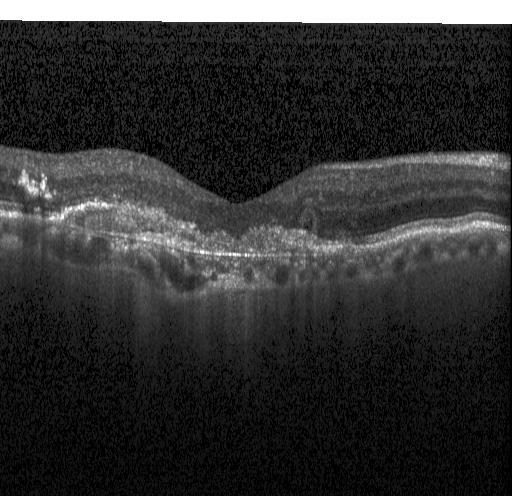

OCT line scan. Centered on the fovea
The scan shows a choroidal neovascular membrane.